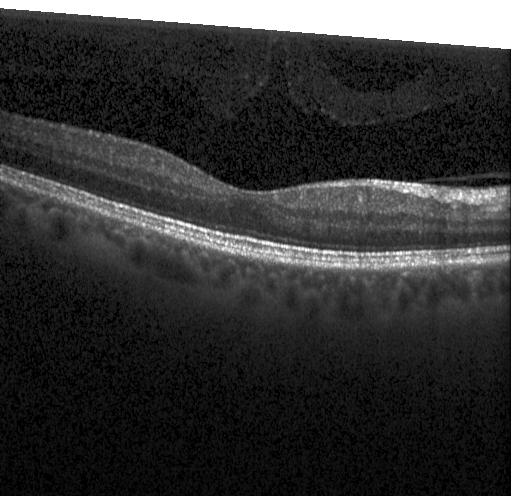

Spectral-domain optical coherence tomography, OCT line scan, horizontal scan through the fovea.
Impression: no CNV, no DME, and no drusen.